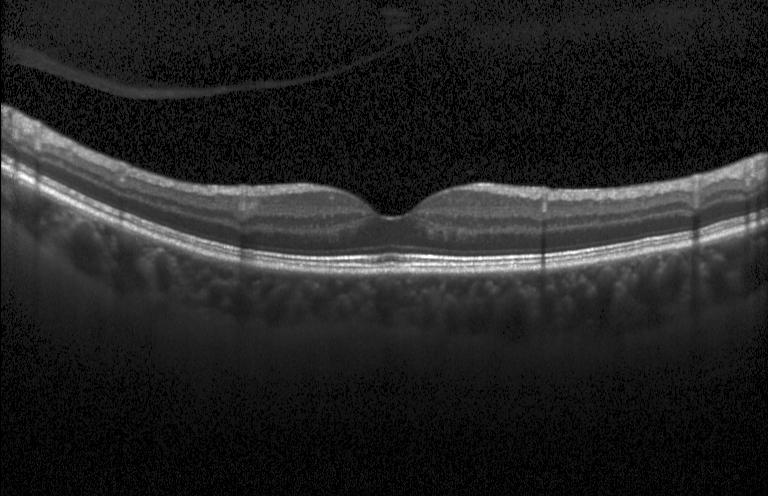 Macular scan, SD-OCT, OCT B-scan
Diagnosis: neither choroidal neovascularization, diabetic macular edema, nor drusen.